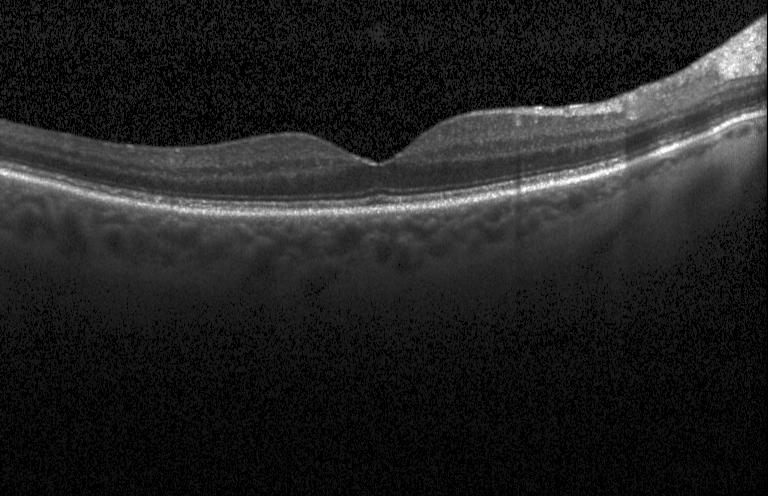 OCT line scan. Instrument: Heidelberg Spectralis. Spectral-domain OCT.
Macular OCT: neither choroidal neovascularization, diabetic macular edema, nor drusen.